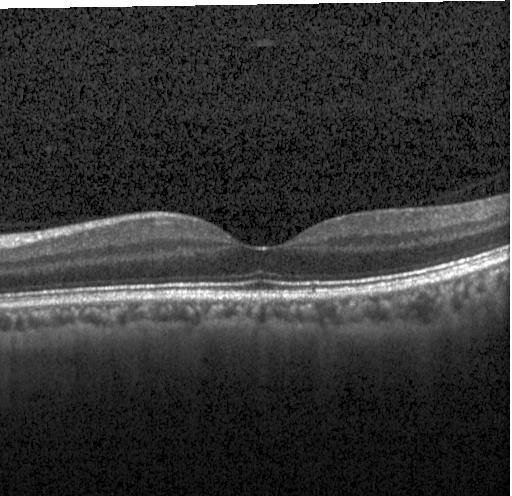 Retinal OCT B-scan · Heidelberg Spectralis. Assessment: no choroidal neovascularization, diabetic macular edema, or drusen.